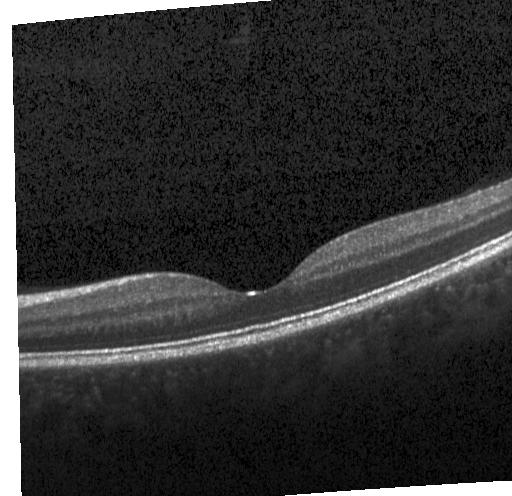 Optical coherence tomography B-scan. Spectral-domain optical coherence tomography. Finding: no choroidal neovascularization, diabetic macular edema, or drusen.